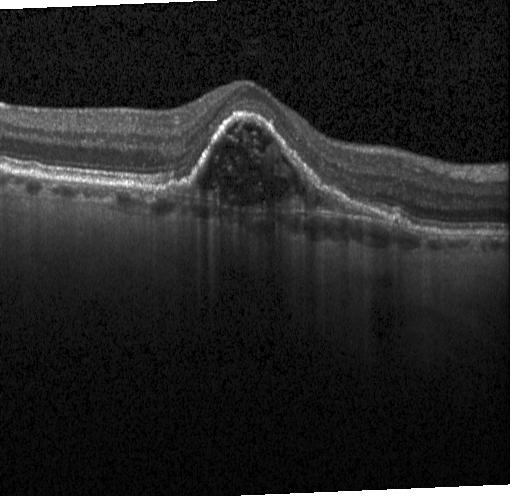
OCT finding: a choroidal neovascular membrane.